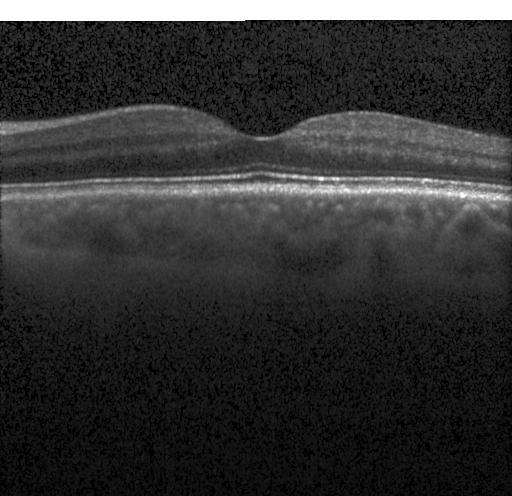 Retinal OCT B-scan. Assessment: no evidence of choroidal neovascularization, diabetic macular edema, or drusen.